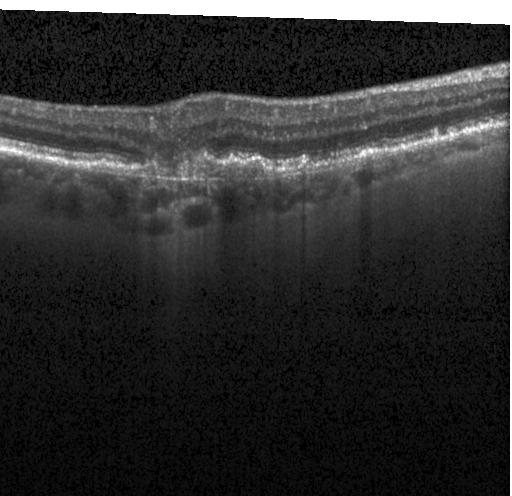

OCT scan showing CNV.